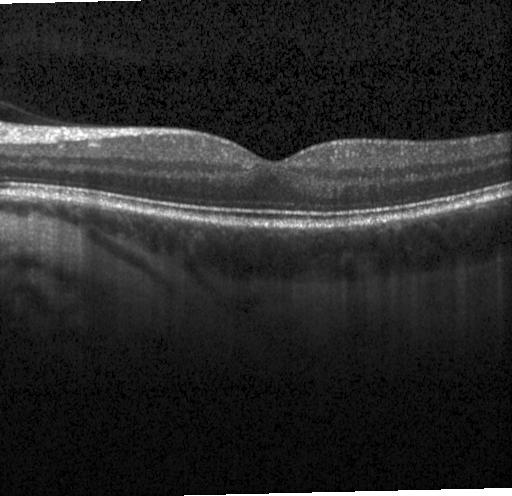 The scan shows no evidence of choroidal neovascularization, diabetic macular edema, or drusen.